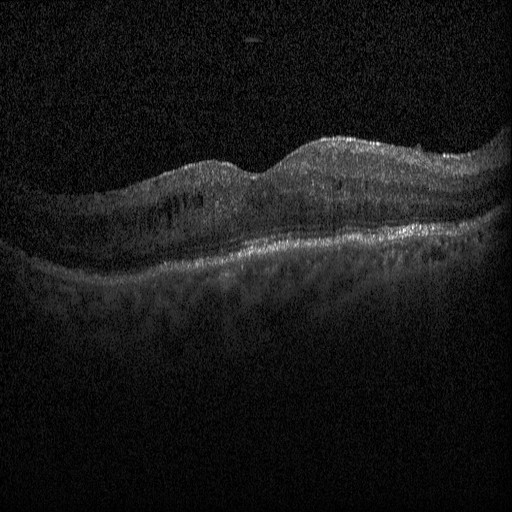

Retinal OCT cross-section; Heidelberg Spectralis — Finding: DME.